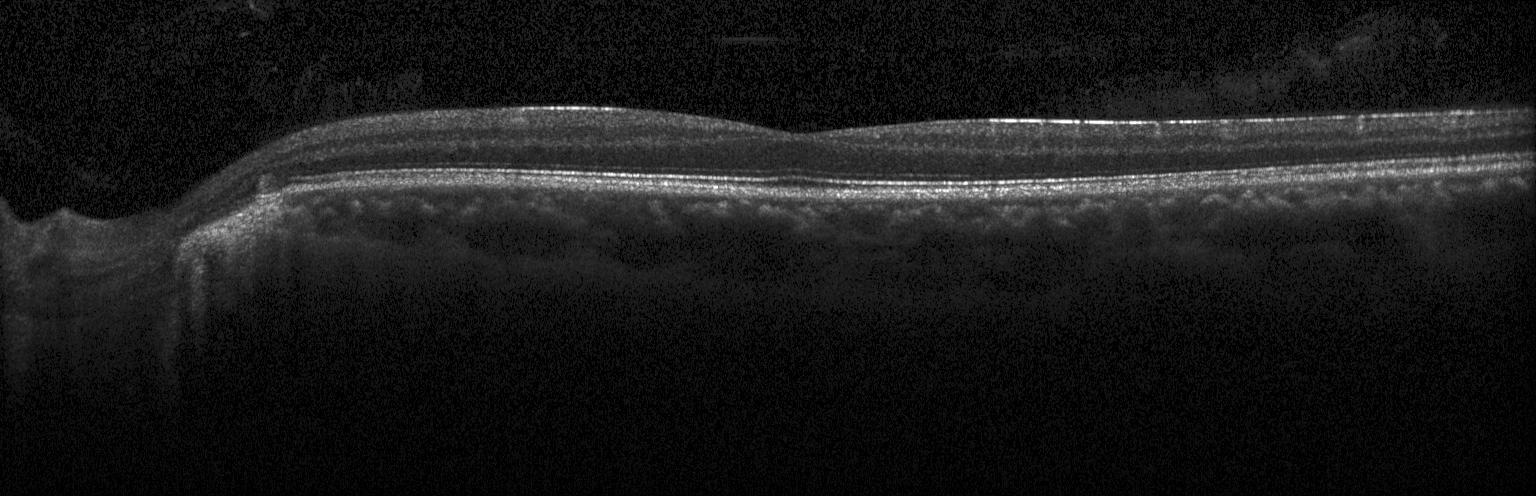

Instrument: Heidelberg Spectralis; spectral-domain optical coherence tomography; OCT line scan. The scan shows no choroidal neovascularization, diabetic macular edema, or drusen.